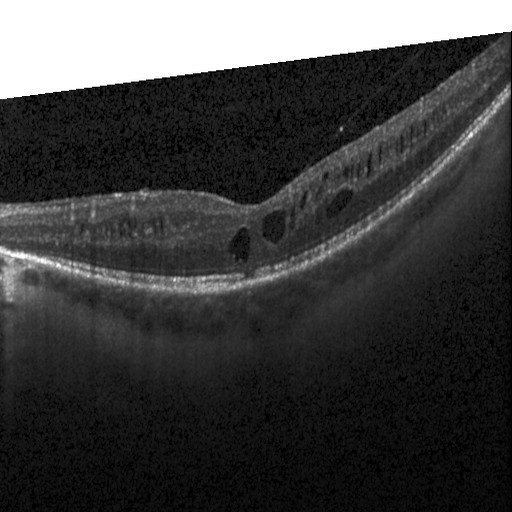

The scan shows DME.